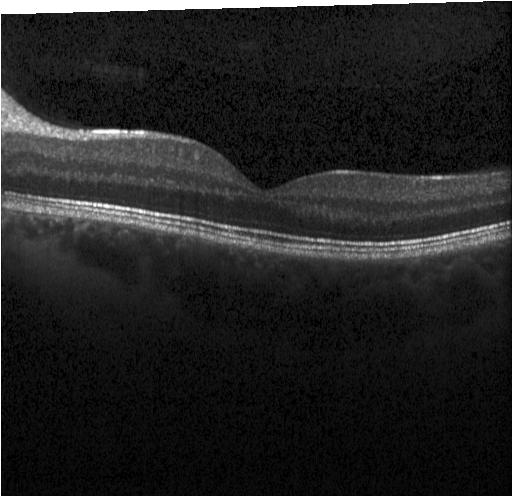 Horizontal scan through the fovea. OCT line scan. Heidelberg Spectralis OCT system. Spectral-domain optical coherence tomography
Finding: no evidence of choroidal neovascularization, diabetic macular edema, or drusen.